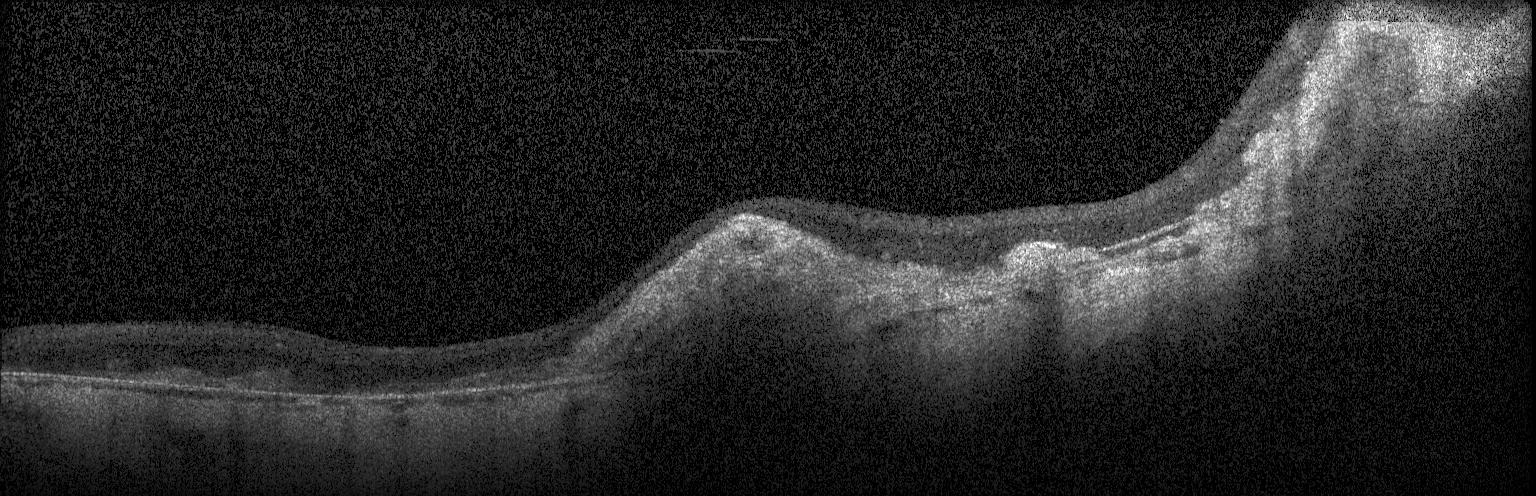

Retinal OCT cross-section. Finding: choroidal neovascularization.